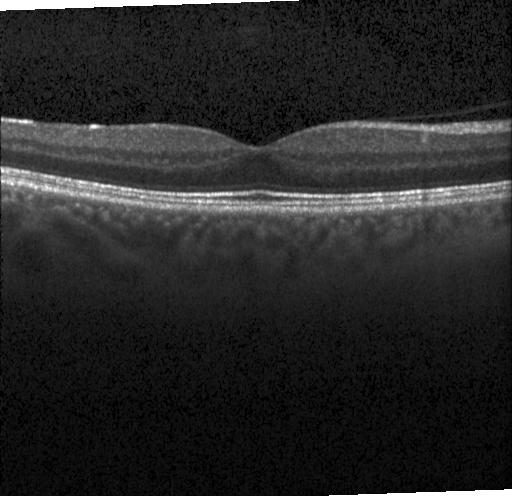

Impression: no evidence of choroidal neovascularization, diabetic macular edema, or drusen.